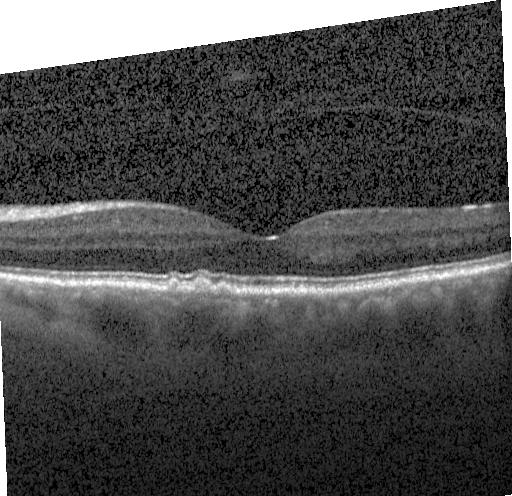
Diagnosis: sub-RPE drusenoid deposits.